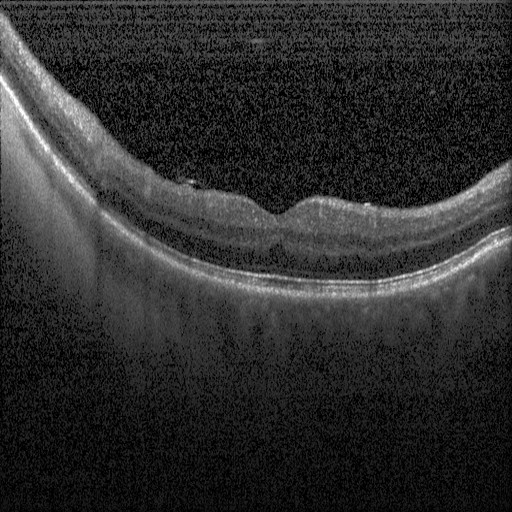 OCT B-scan; acquired on a Heidelberg Spectralis — Finding: diabetic macular edema (DME).